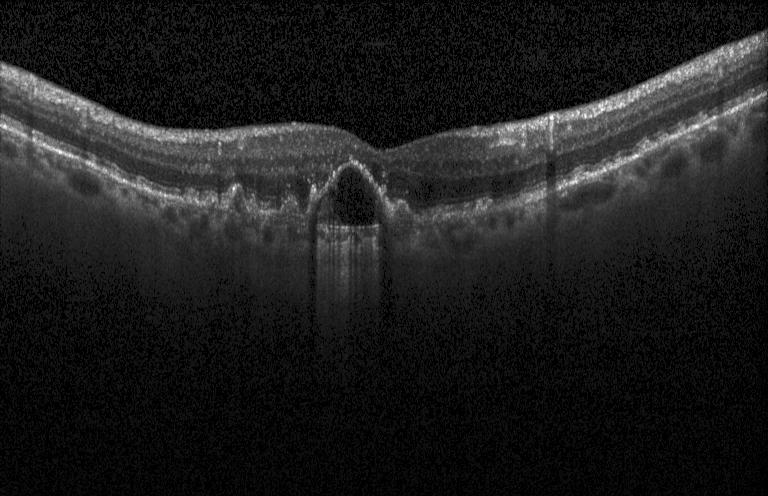

Heidelberg Spectralis OCT system, SD-OCT, optical coherence tomography scan, through the macula — Choroidal neovascularization.